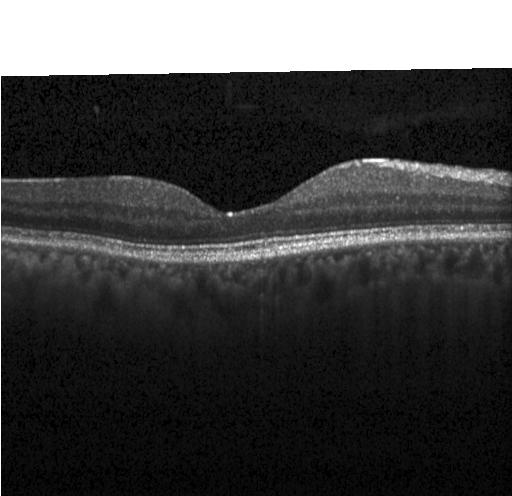
Finding: neither choroidal neovascularization, diabetic macular edema, nor drusen.